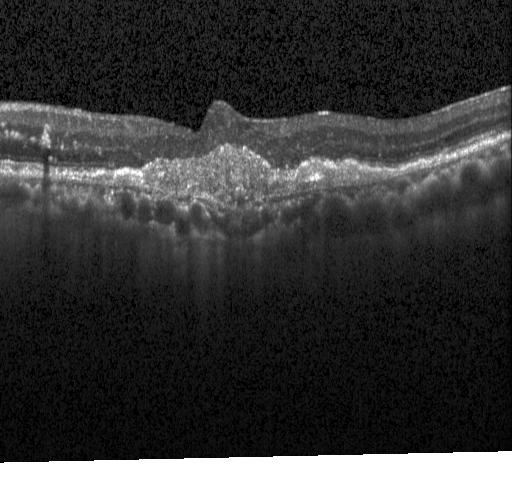
Retinal OCT cross-section; through the macula; Heidelberg Spectralis OCT system; SD-OCT. Assessment: a choroidal neovascular membrane.